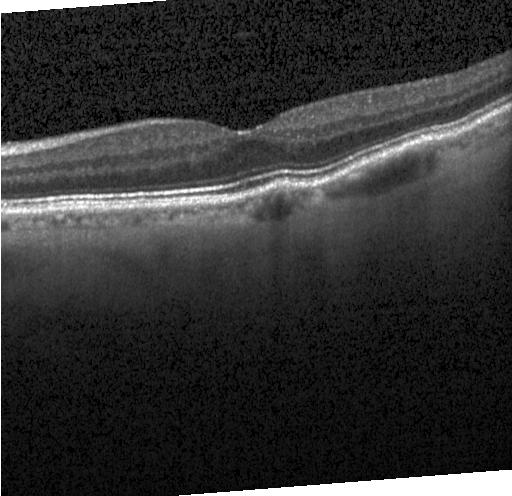

Optical coherence tomography B-scan; SD-OCT; horizontal scan through the fovea; acquired on a Heidelberg Spectralis.
Assessment: no evidence of choroidal neovascularization, diabetic macular edema, or drusen.